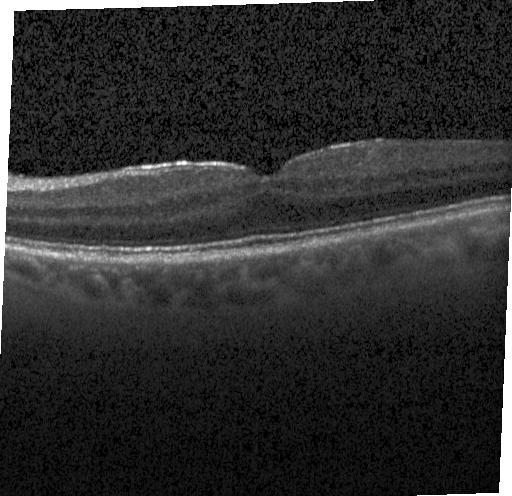 Diagnosis: neither choroidal neovascularization, diabetic macular edema, nor drusen.